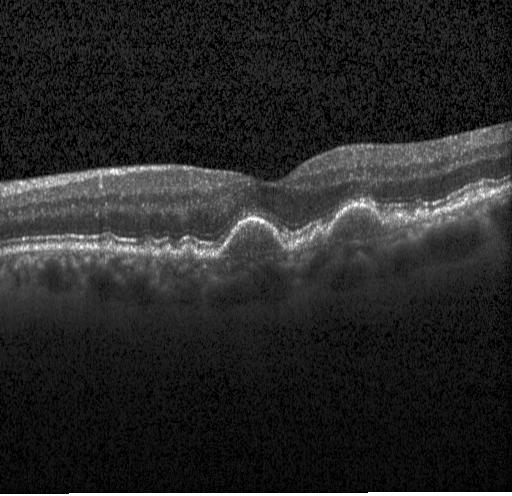
Diagnosis: multiple drusen.